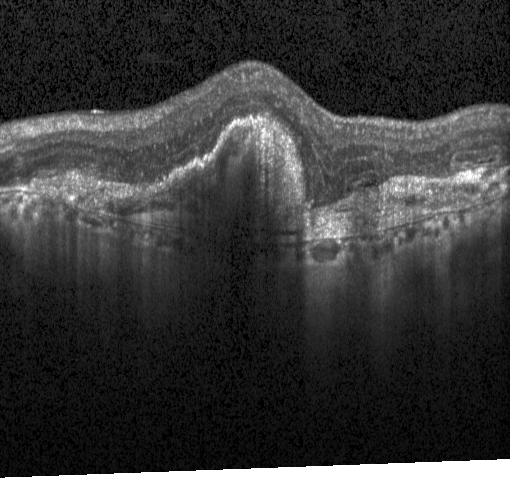 Heidelberg Spectralis OCT system. Retinal OCT B-scan — A choroidal neovascular membrane.